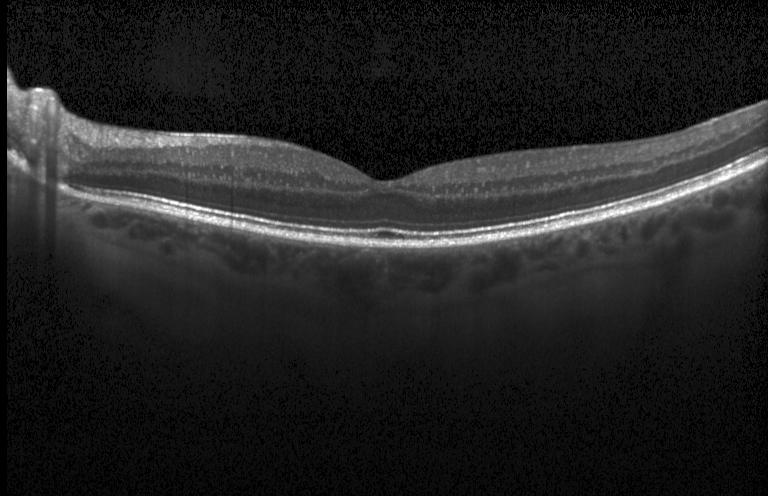 Finding: no evidence of choroidal neovascularization, diabetic macular edema, or drusen.